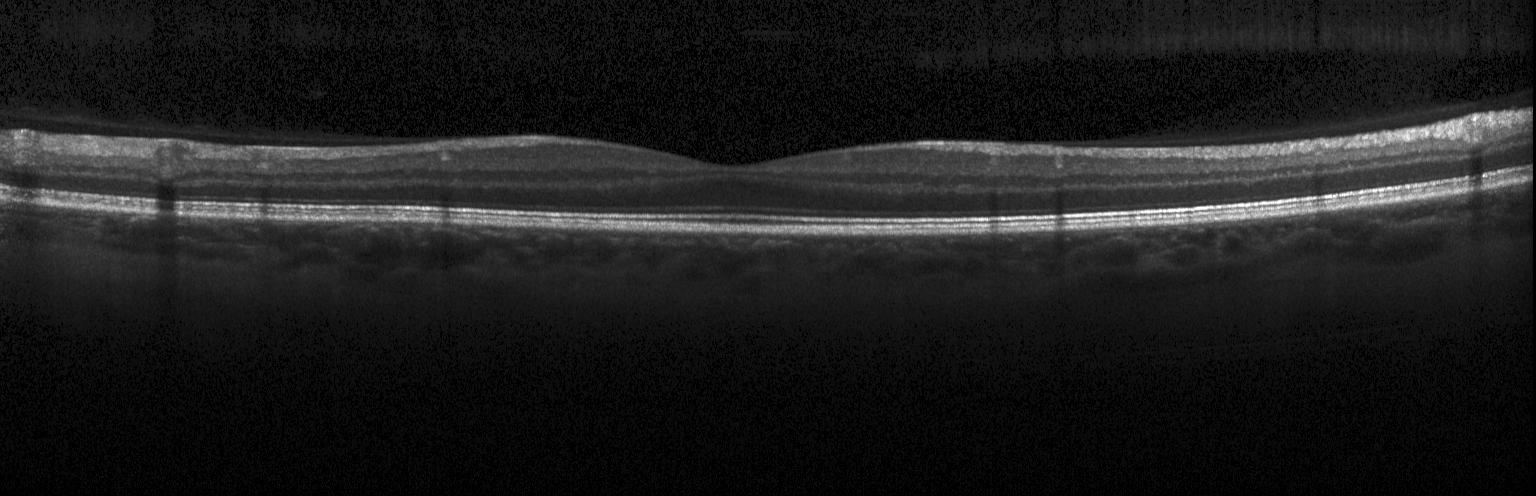
Optical coherence tomography scan · centered on the fovea · spectral-domain OCT
Impression: no evidence of CNV, DME, or drusen.